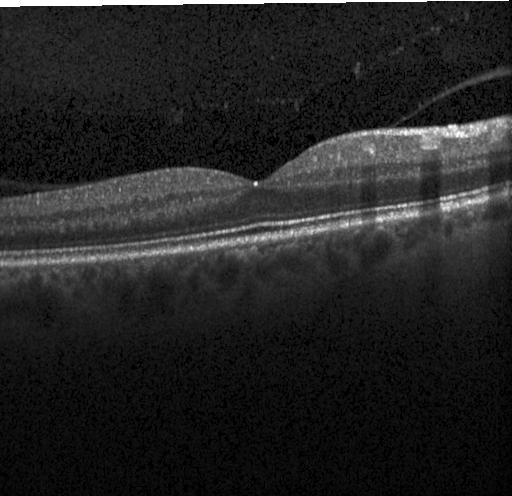

Retinal OCT cross-section.
Impression: neither choroidal neovascularization, diabetic macular edema, nor drusen.